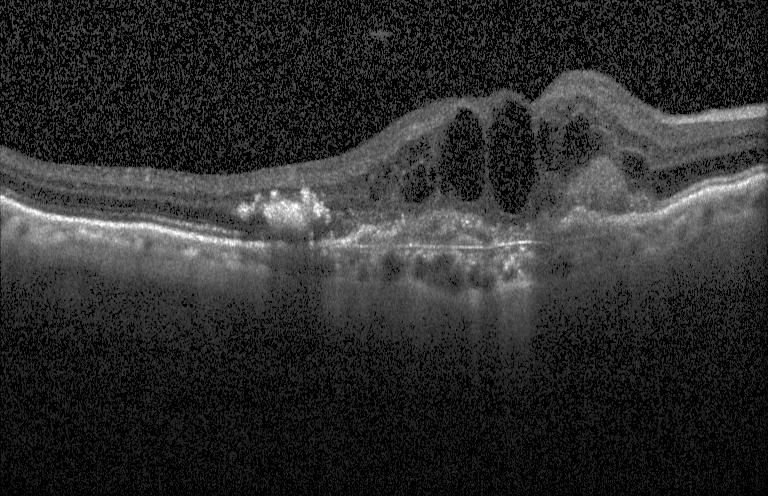 Retinal OCT cross-section
Impression: a choroidal neovascular membrane.